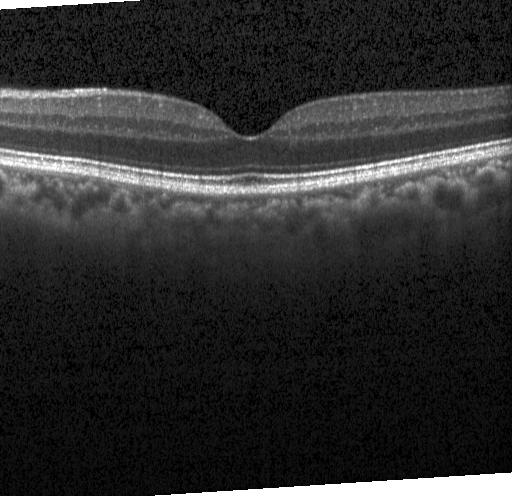
Optical coherence tomography scan · horizontal scan through the fovea · Heidelberg Spectralis OCT system. This B-scan demonstrates no choroidal neovascularization, diabetic macular edema, or drusen.